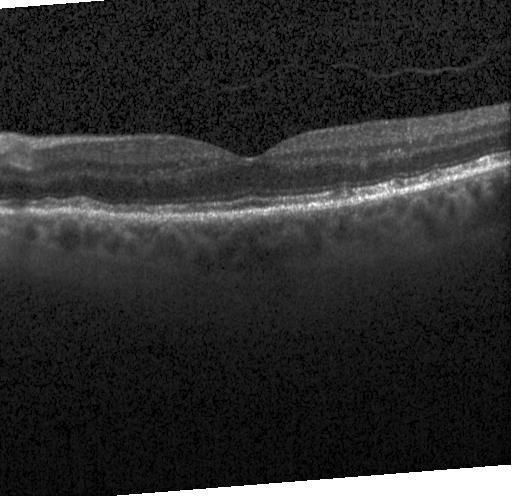 Impression: drusen.